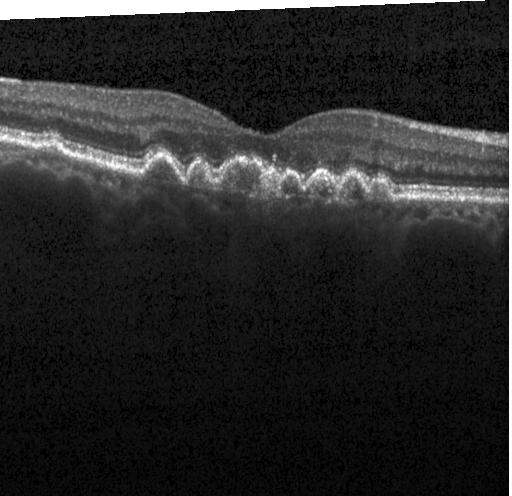
The scan shows sub-RPE drusenoid deposits.